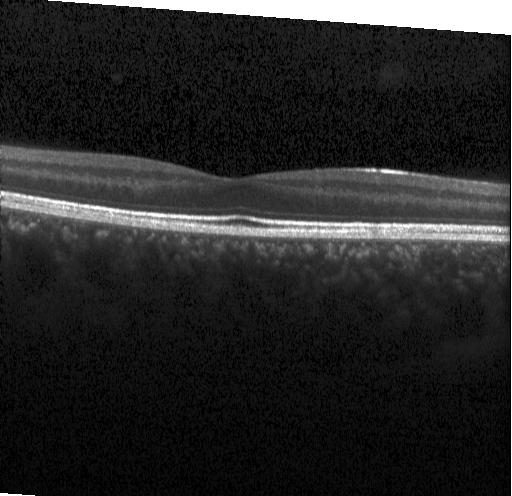
Spectral-domain OCT. OCT B-scan — Macular OCT: no evidence of choroidal neovascularization, diabetic macular edema, or drusen.